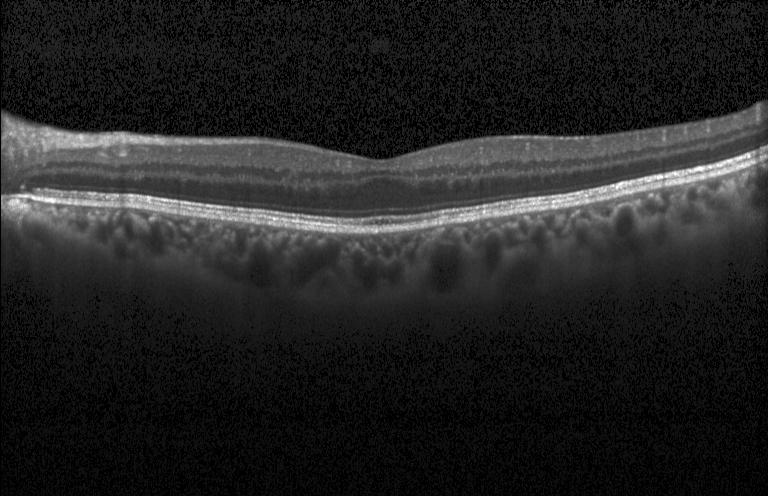
Diagnosis: neither choroidal neovascularization, diabetic macular edema, nor drusen.